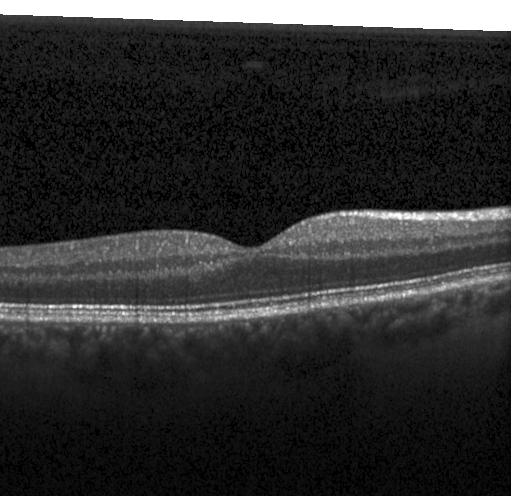
Dx: no evidence of choroidal neovascularization, diabetic macular edema, or drusen.